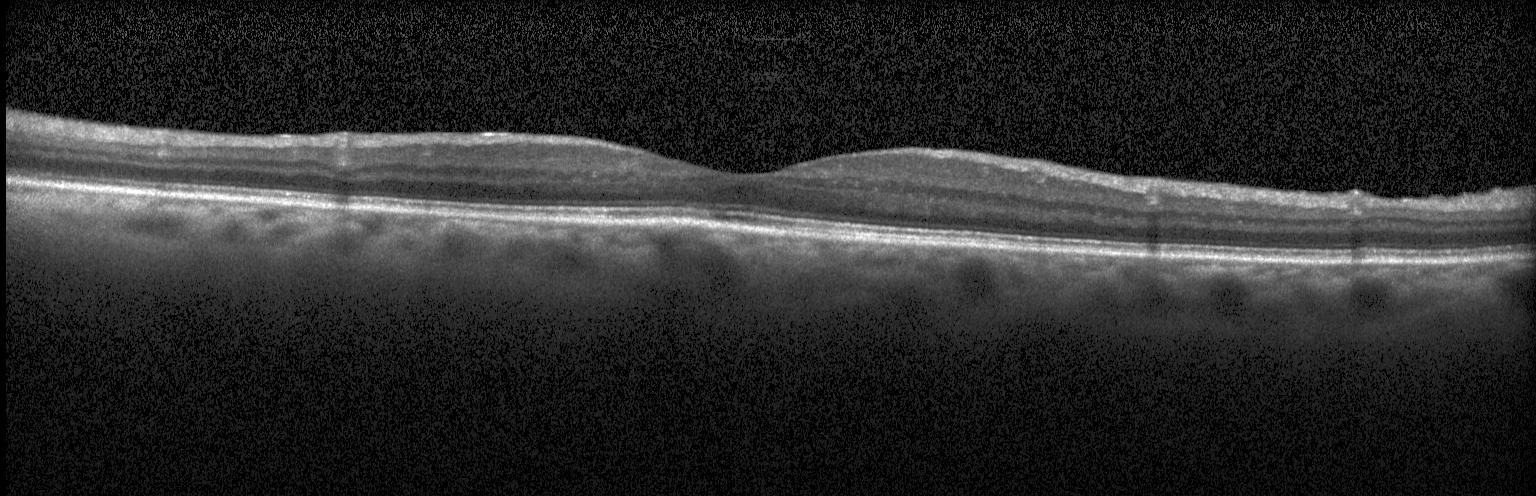
OCT scan showing no evidence of choroidal neovascularization, diabetic macular edema, or drusen.